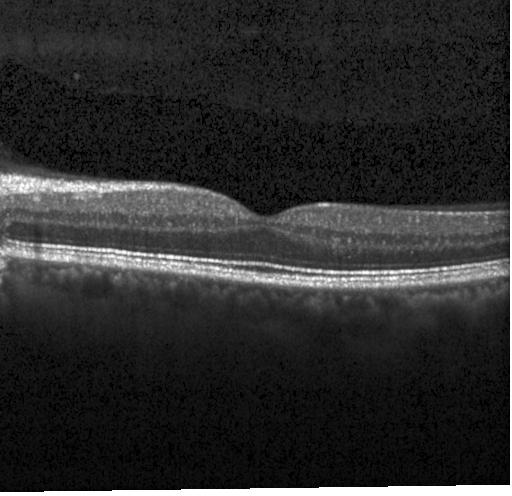 Optical coherence tomography B-scan
Impression: no evidence of CNV, DME, or drusen.